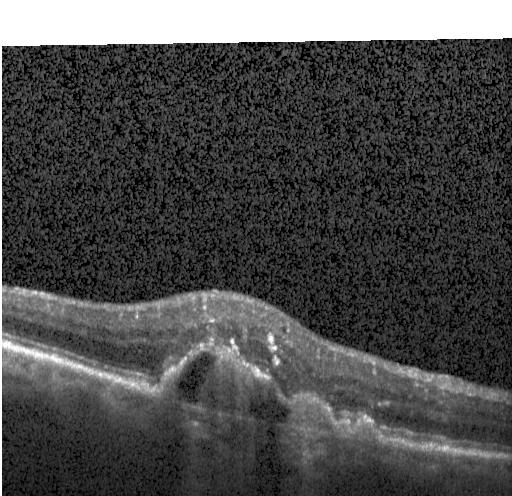 Finding: a choroidal neovascular membrane.